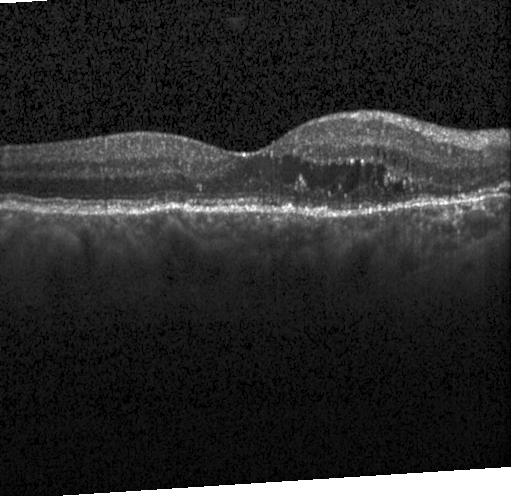

OCT scan showing diabetic macular edema.